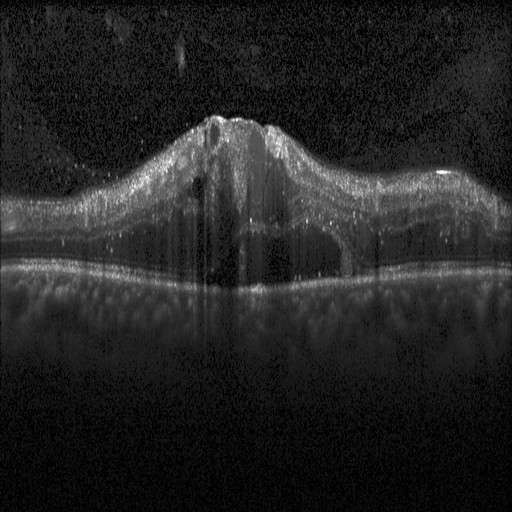
Dx: diabetic macular edema.